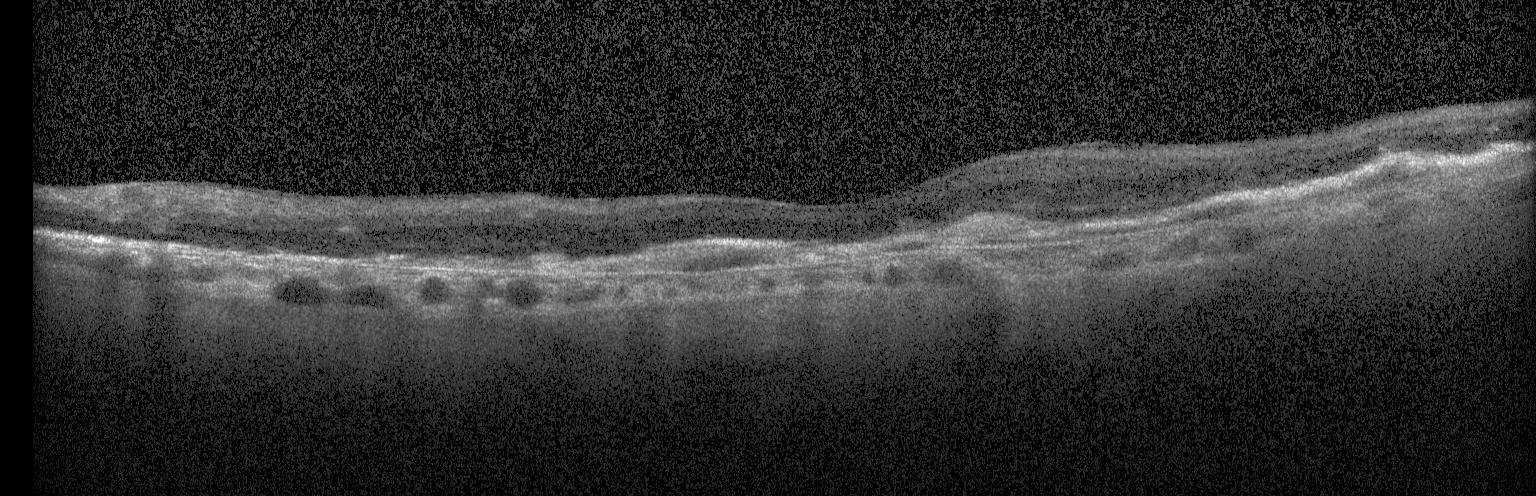

Spectral-domain OCT B-scan: CNV.